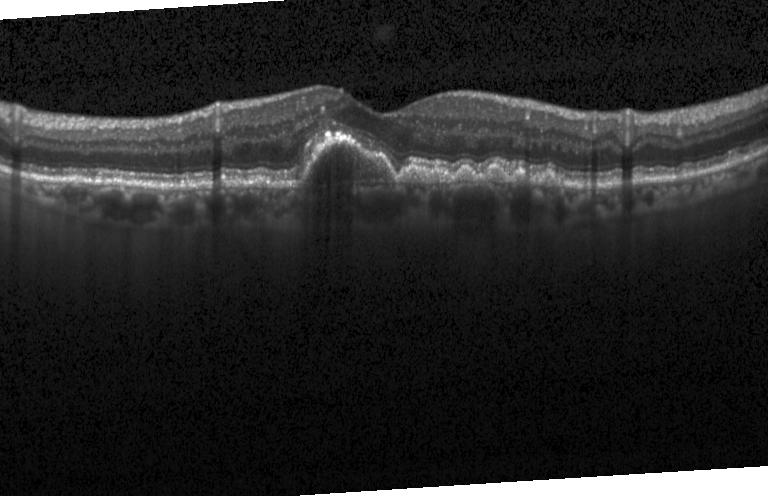

Impression: multiple drusen.